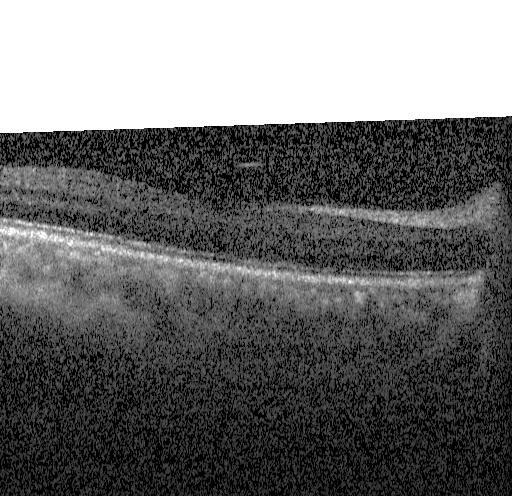

No evidence of choroidal neovascularization, diabetic macular edema, or drusen.